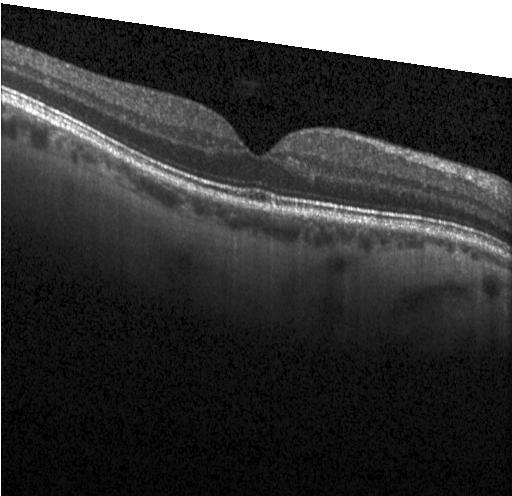

Diagnosis: neither CNV, DME, nor drusen.